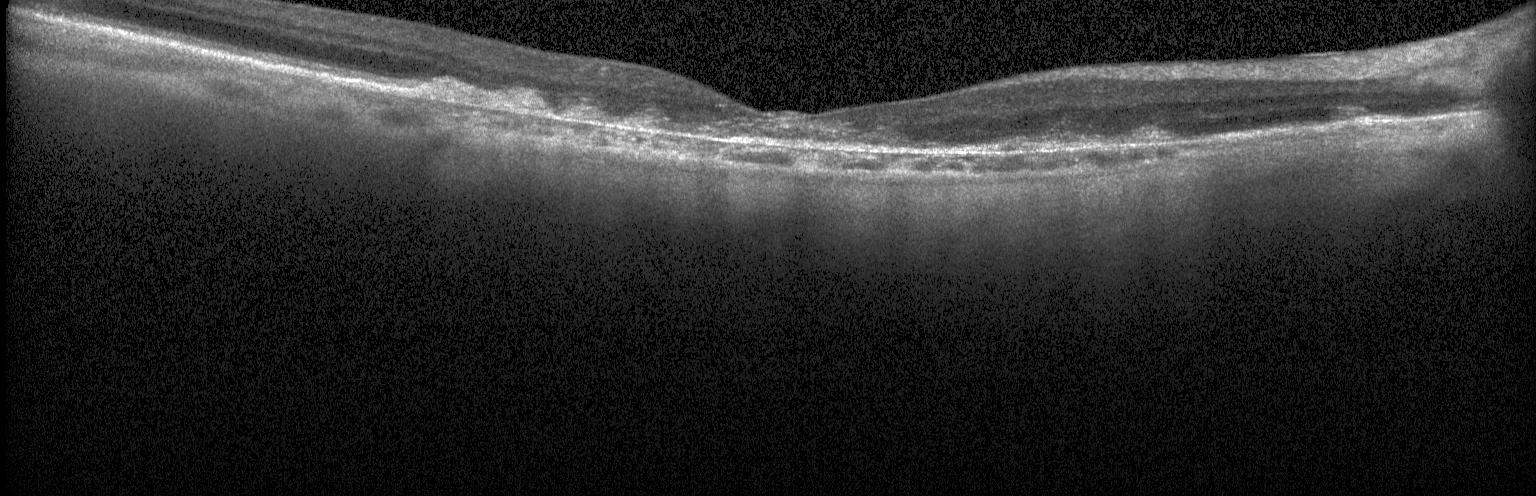
Finding: a choroidal neovascular membrane.